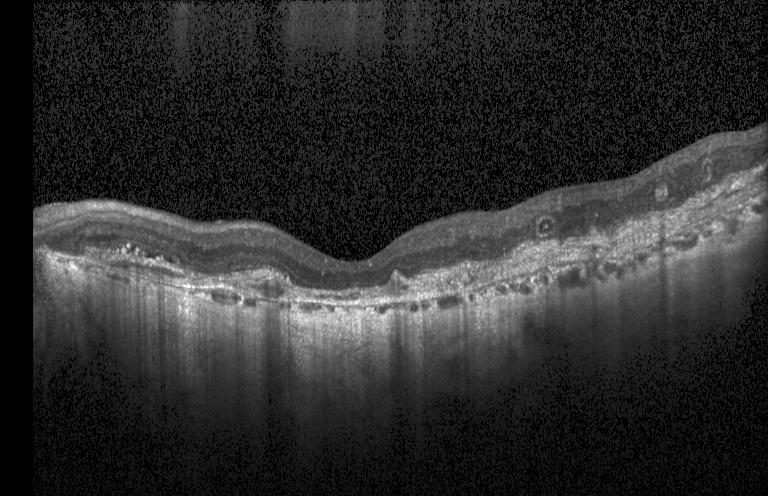 OCT finding: a choroidal neovascular membrane.